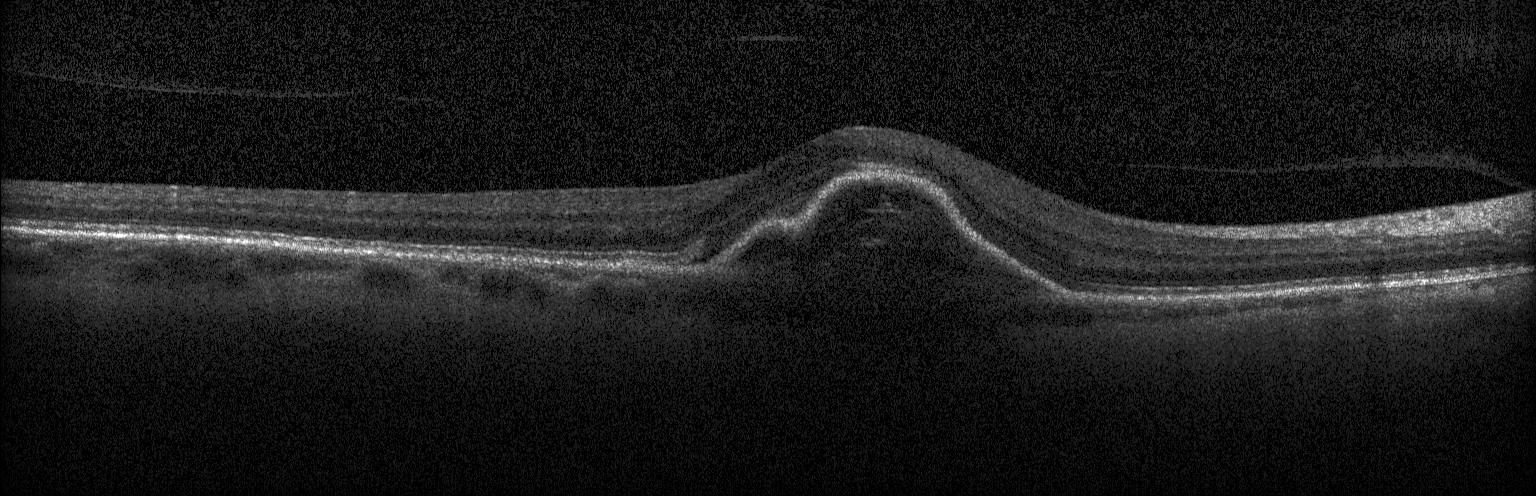 Macular OCT demonstrating choroidal neovascularization (CNV).